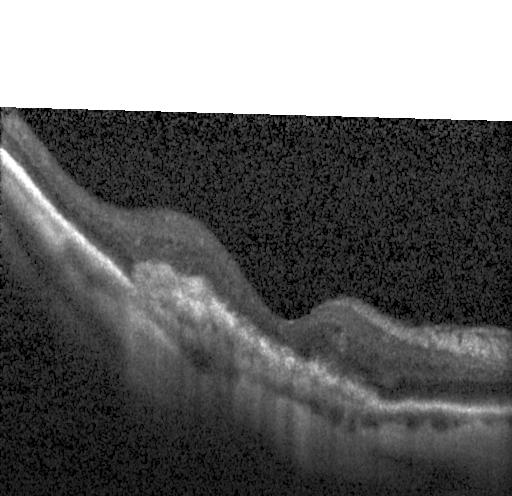

Impression: CNV.